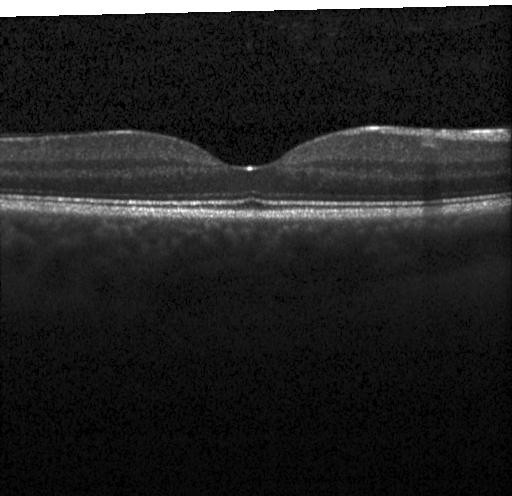

OCT line scan. Spectral-domain OCT
Neither CNV, DME, nor drusen.